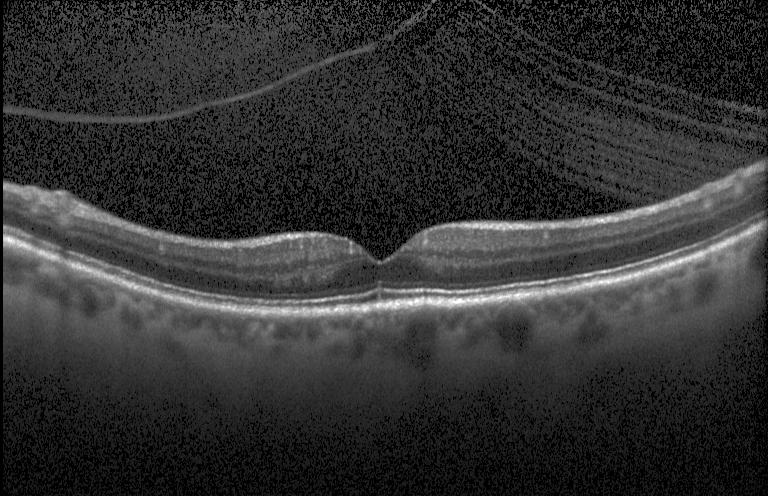
Macular OCT: no choroidal neovascularization, no diabetic macular edema, and no drusen.